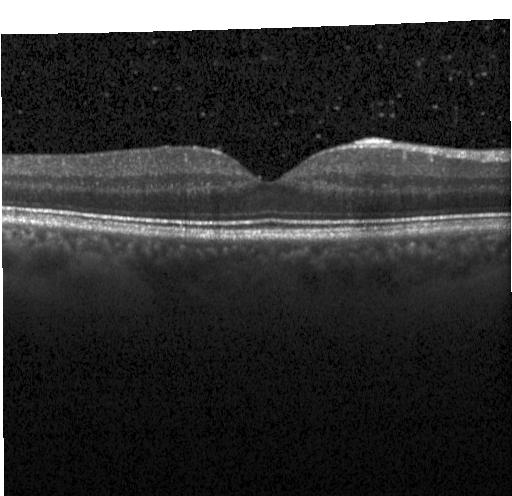

Optical coherence tomography scan · through the macula · spectral-domain optical coherence tomography — Diagnosis: no evidence of choroidal neovascularization, diabetic macular edema, or drusen.